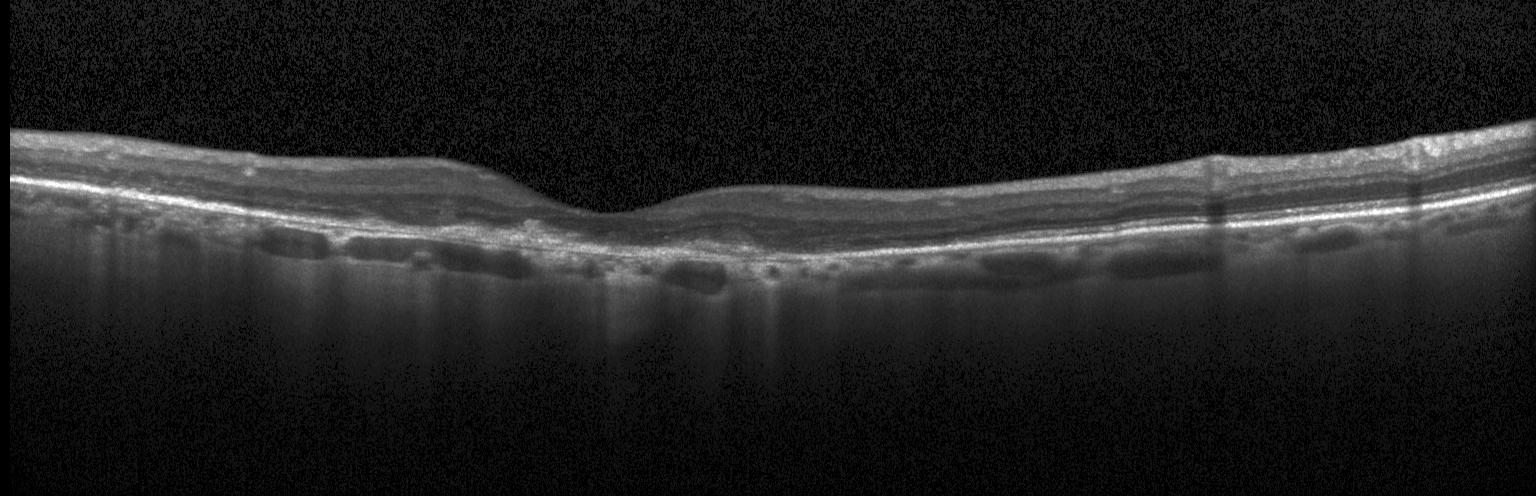 A choroidal neovascular membrane.